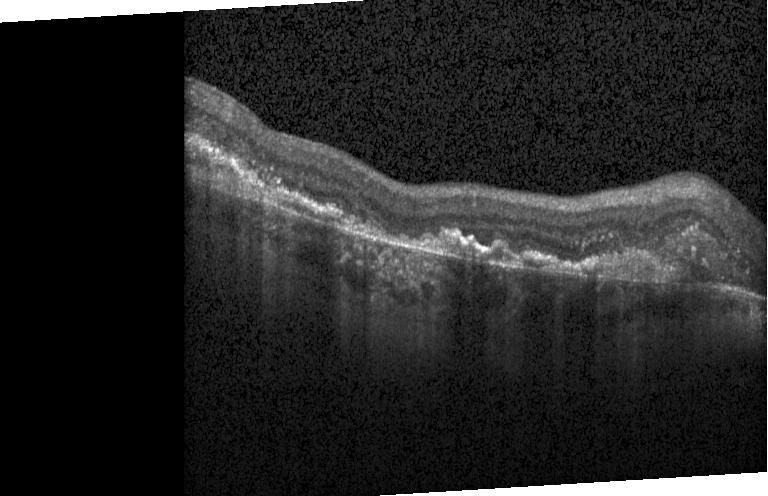

OCT B-scan showing a choroidal neovascular membrane.